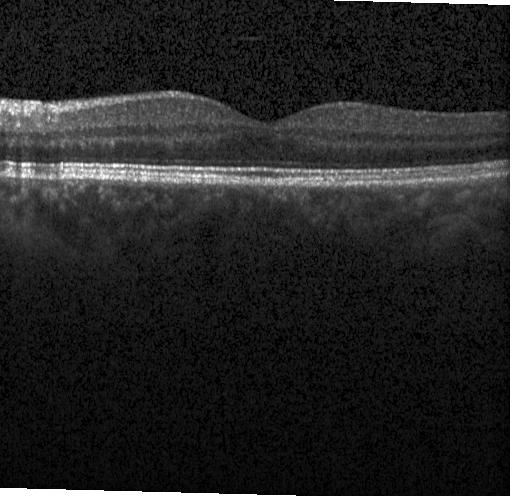

This B-scan demonstrates no CNV, no DME, and no drusen.